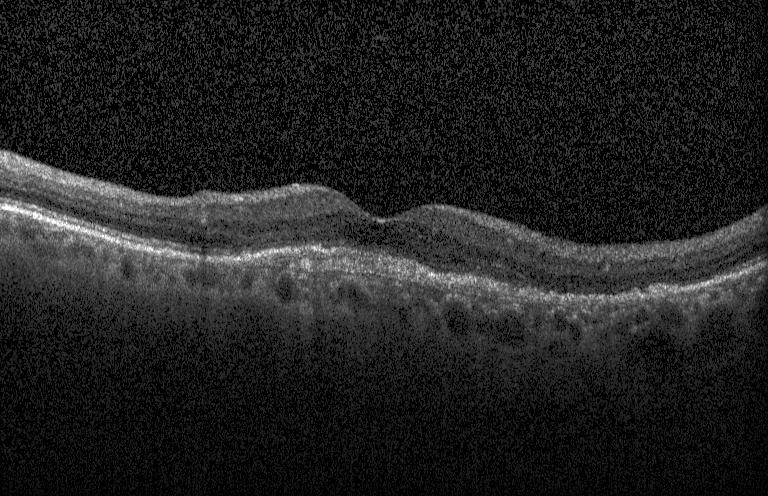
Optical coherence tomography B-scan.
Finding: a choroidal neovascular membrane.